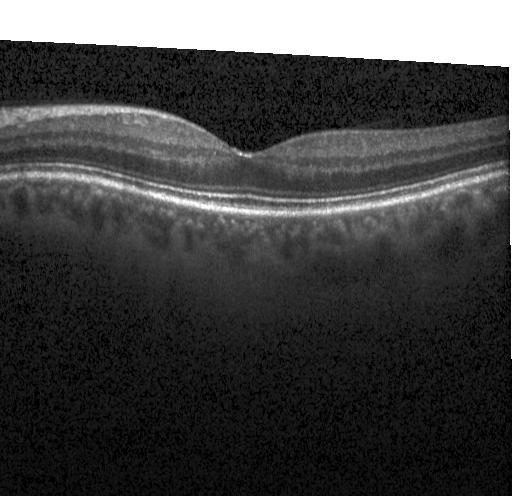
Impression: no evidence of choroidal neovascularization, diabetic macular edema, or drusen.